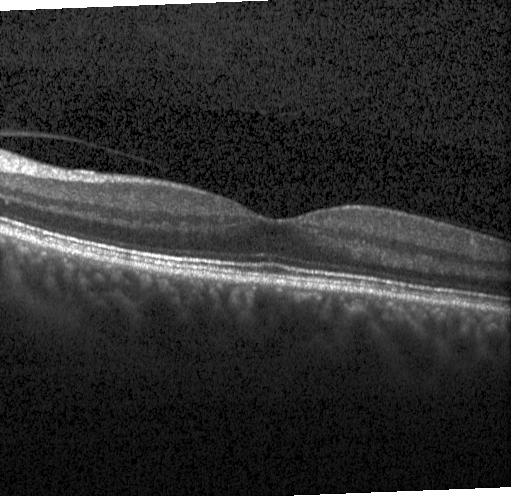

Macular OCT demonstrating neither choroidal neovascularization, diabetic macular edema, nor drusen.